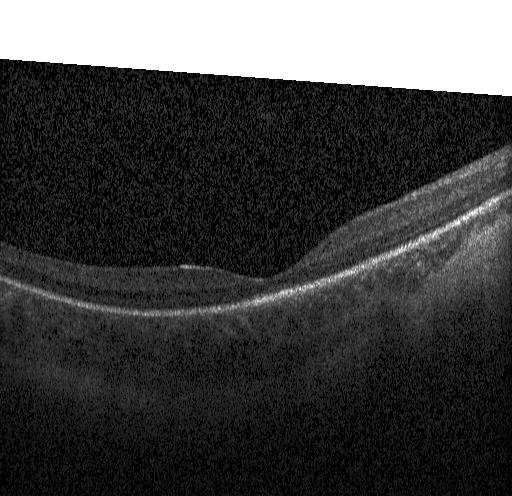
The scan shows no choroidal neovascularization, no diabetic macular edema, and no drusen.